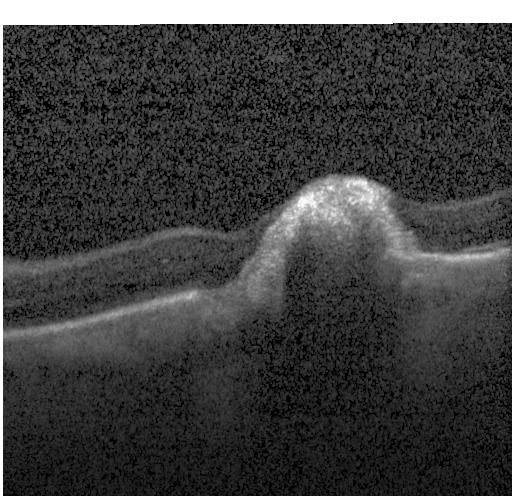

OCT line scan; acquired on a Heidelberg Spectralis; SD-OCT.
This B-scan demonstrates a choroidal neovascular membrane.